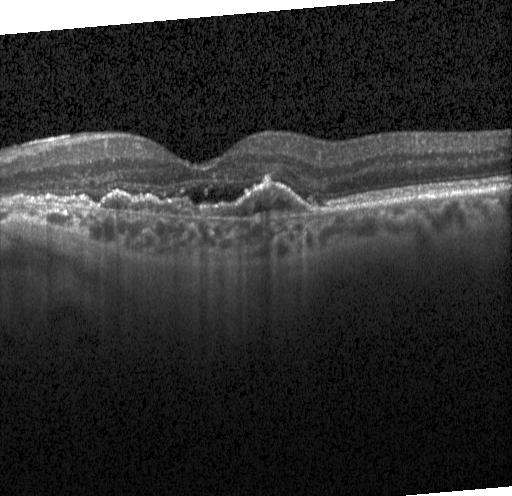 OCT B-scan showing choroidal neovascularization.